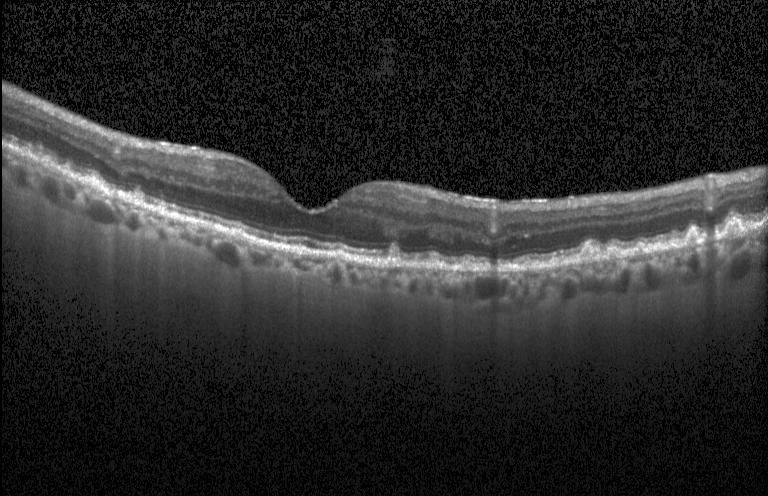
Retinal OCT B-scan. Through the macula. Acquired on a Heidelberg Spectralis. Spectral-domain OCT.
OCT finding: sub-RPE drusenoid deposits.